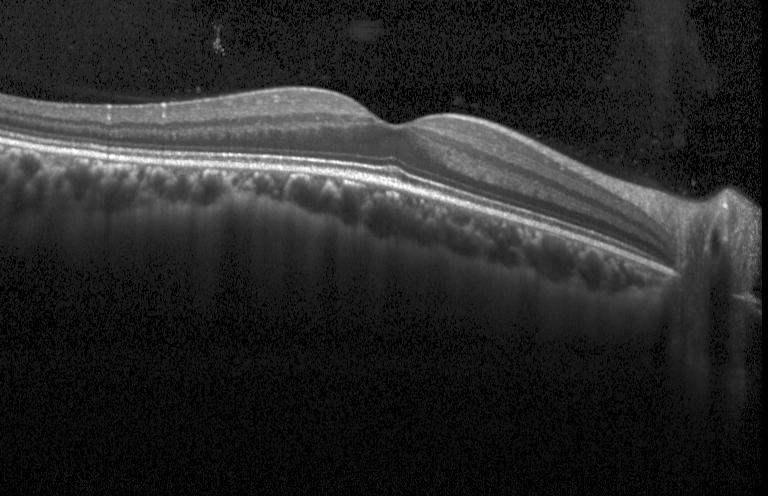
Acquired on a Heidelberg Spectralis; retinal OCT B-scan; spectral-domain OCT; centered on the fovea — Diagnosis: no choroidal neovascularization, diabetic macular edema, or drusen.